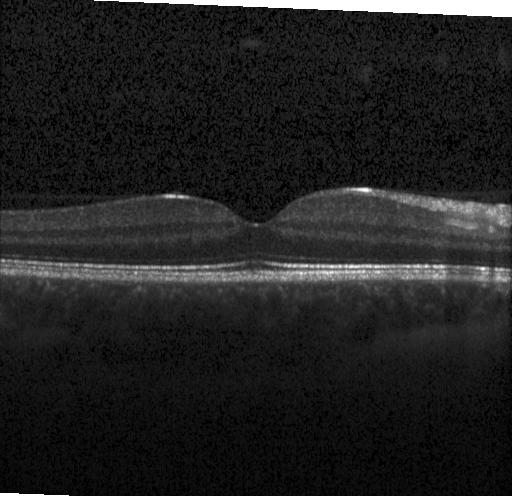
OCT line scan · spectral-domain OCT. This B-scan demonstrates neither CNV, DME, nor drusen.